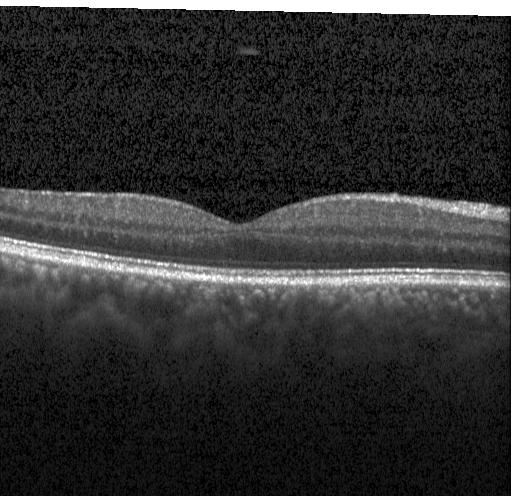 Retinal OCT cross-section; spectral-domain OCT; Heidelberg Spectralis.
OCT finding: neither choroidal neovascularization, diabetic macular edema, nor drusen.